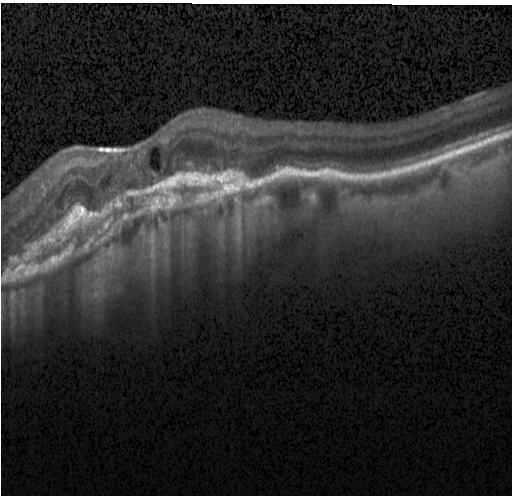 Impression: a choroidal neovascular membrane.